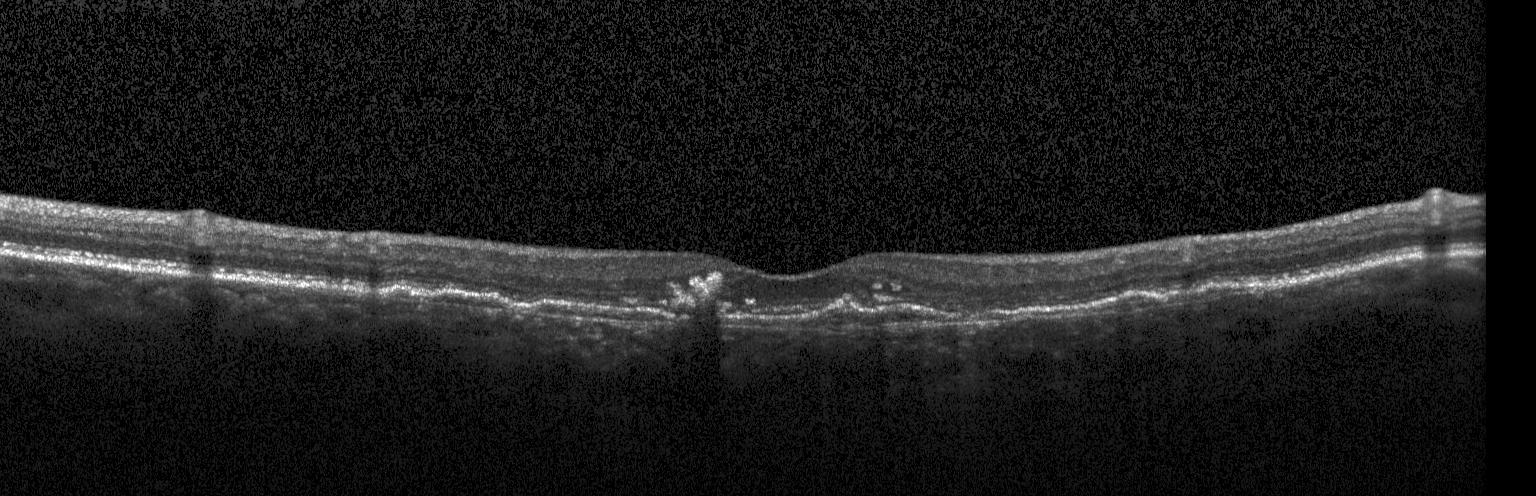
SD-OCT. Heidelberg Spectralis OCT system. Retinal OCT cross-section
Finding: CNV.